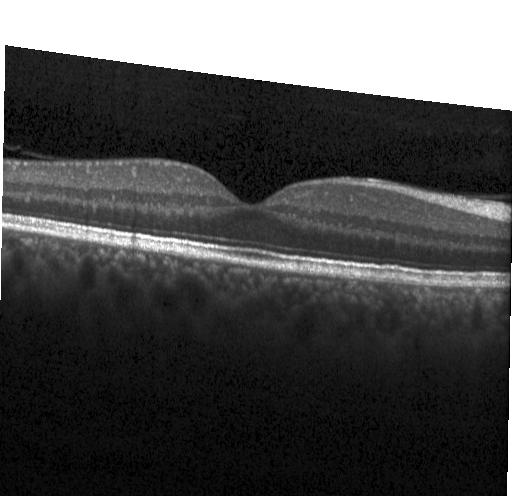 Retinal OCT cross-section; Heidelberg Spectralis OCT system
The scan shows neither choroidal neovascularization, diabetic macular edema, nor drusen.